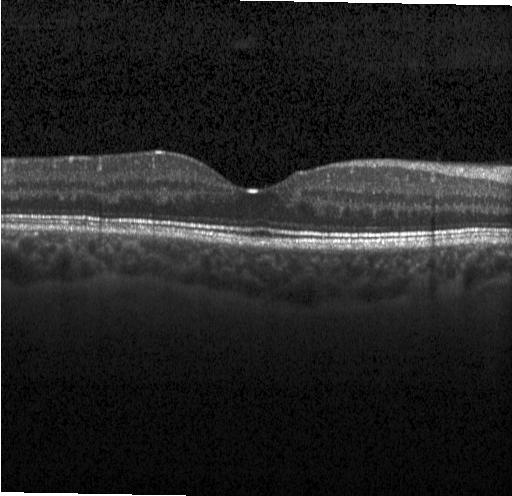
Fovea-centered, Heidelberg Spectralis, OCT line scan. Diagnosis: neither choroidal neovascularization, diabetic macular edema, nor drusen.